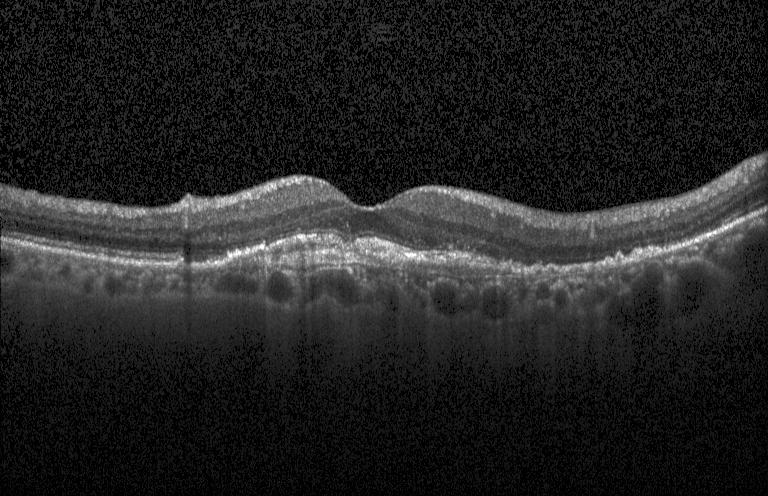 This B-scan demonstrates a choroidal neovascular membrane.